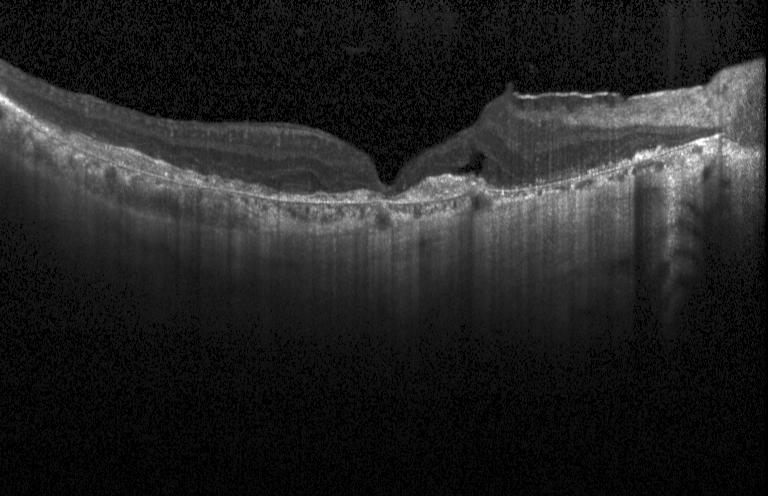
Retinal OCT cross-section
Dx: a choroidal neovascular membrane.